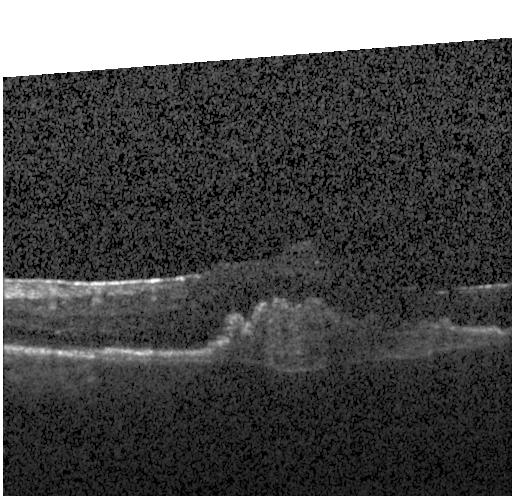 Acquired on a Heidelberg Spectralis. Retinal OCT B-scan. Finding: CNV.